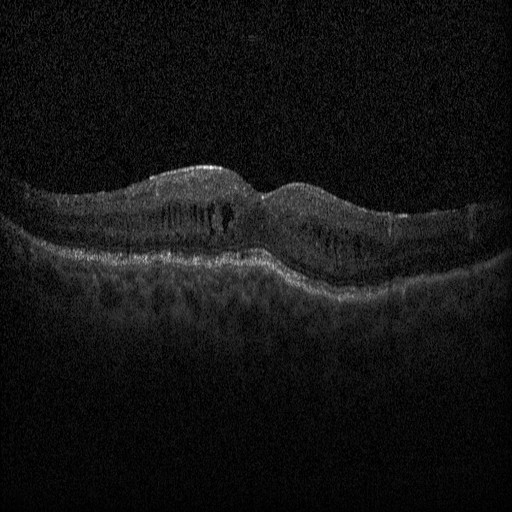

Through the macula; SD-OCT; optical coherence tomography scan; acquired on a Heidelberg Spectralis. Diabetic macular edema.